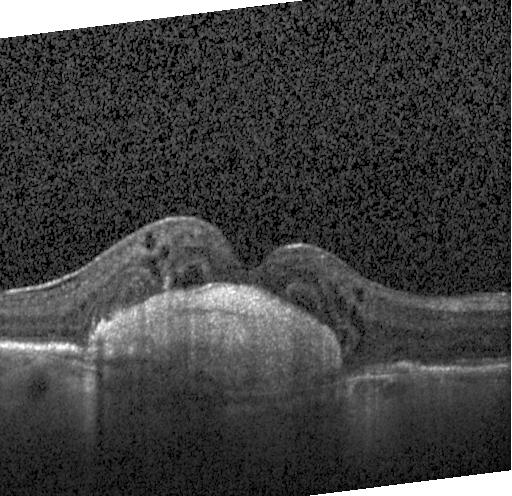 Finding: choroidal neovascularization.